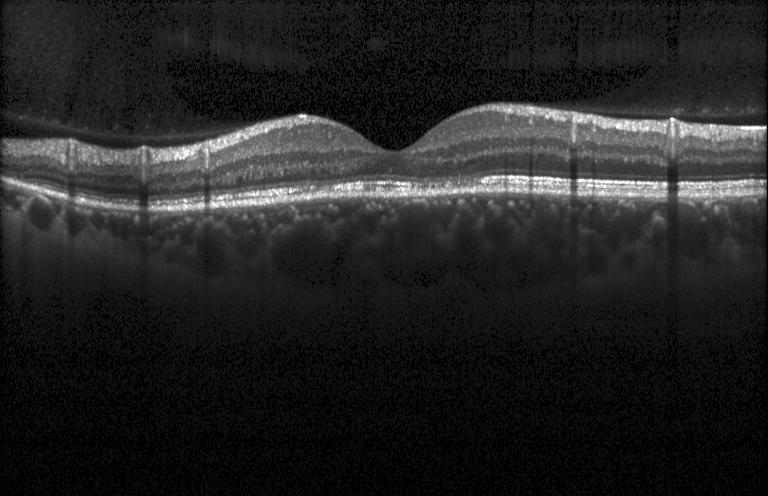 The scan shows no evidence of CNV, DME, or drusen.